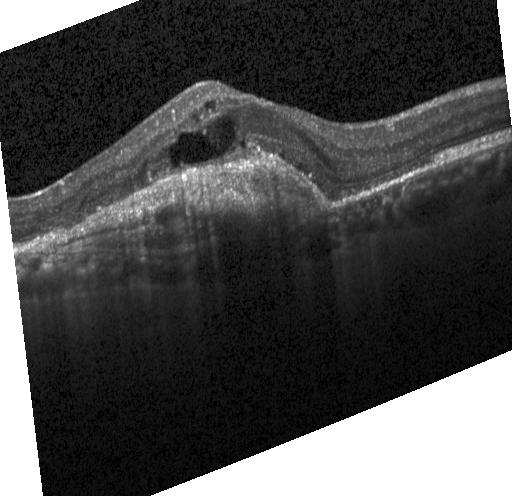 Retinal OCT cross-section. Finding: CNV.